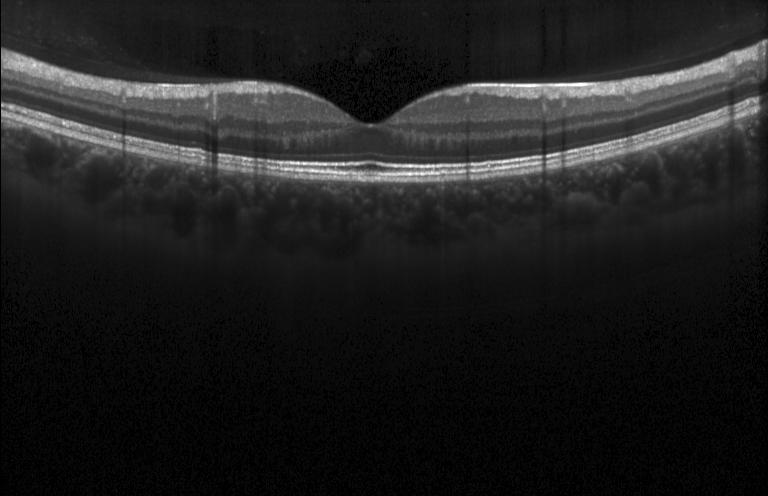 Optical coherence tomography B-scan, macular scan, spectral-domain optical coherence tomography.
Diagnosis: neither CNV, DME, nor drusen.